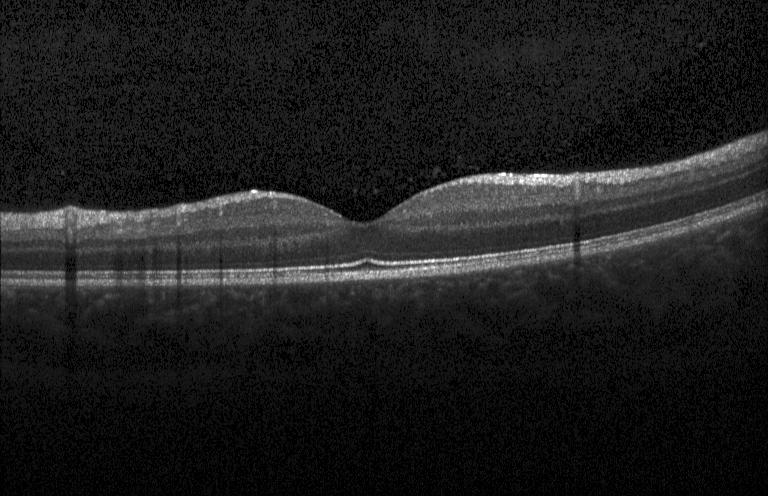

Retinal OCT B-scan
OCT finding: no CNV, DME, or drusen.